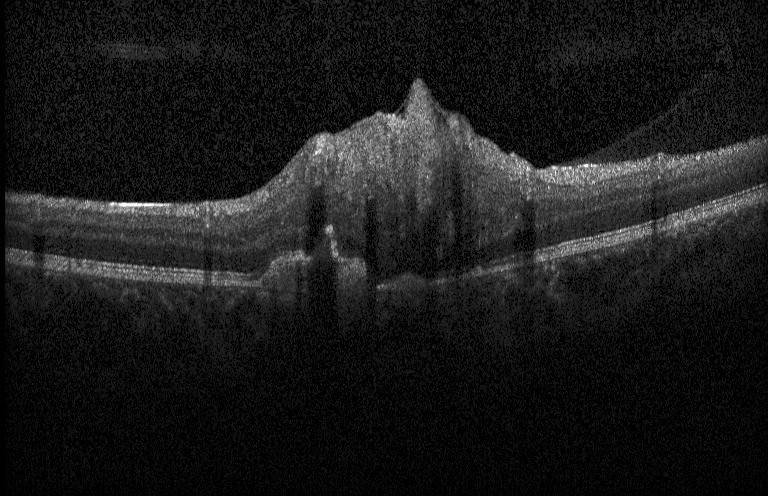 OCT B-scan; spectral-domain optical coherence tomography; macular scan
Impression: a choroidal neovascular membrane.